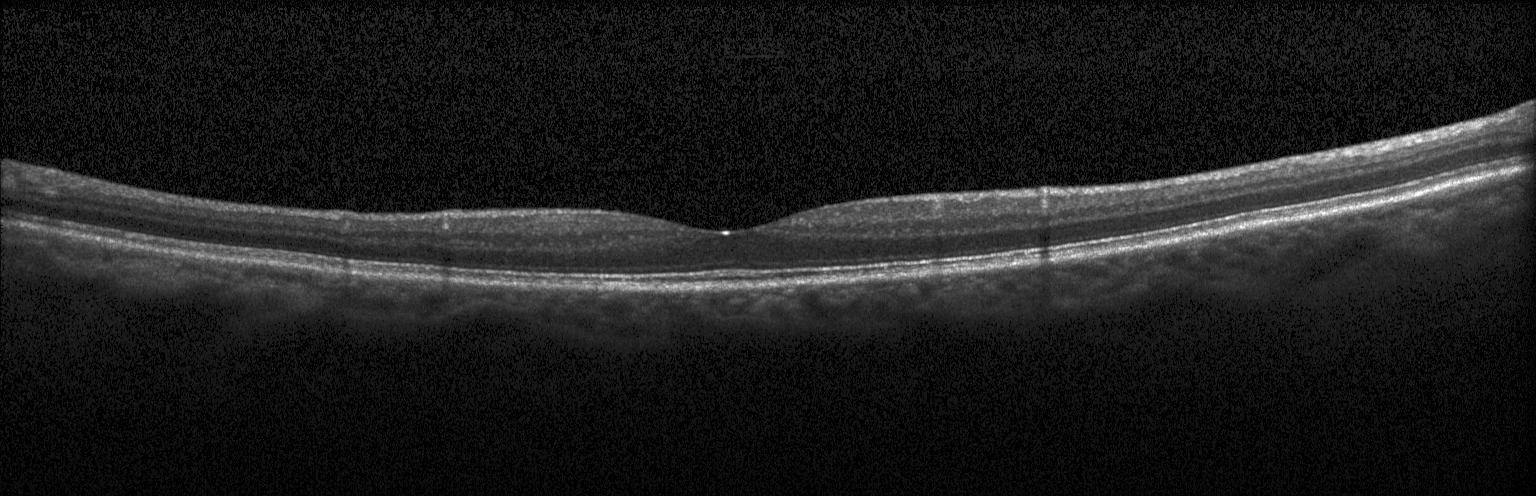
OCT B-scan · acquired on a Heidelberg Spectralis · centered on the fovea — OCT finding: no CNV, no DME, and no drusen.